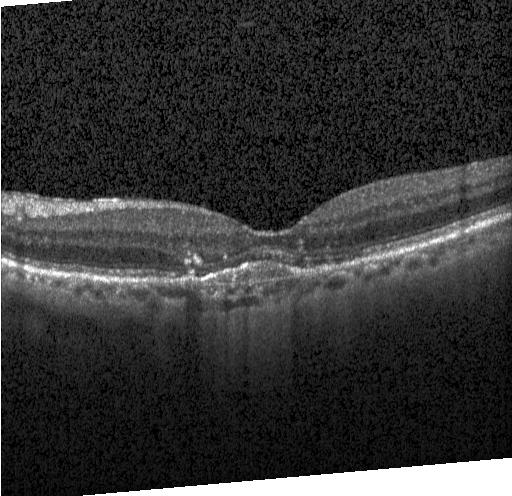 Spectral-domain OCT B-scan: choroidal neovascularization.